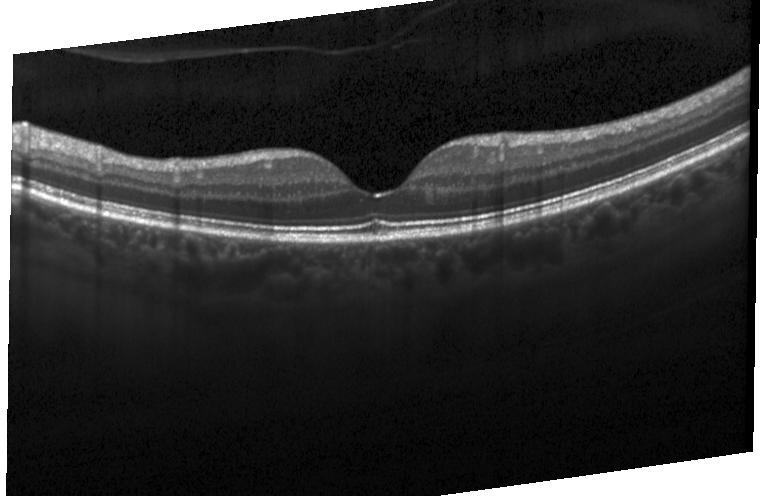

Instrument: Heidelberg Spectralis; OCT B-scan — Impression: no choroidal neovascularization, no diabetic macular edema, and no drusen.